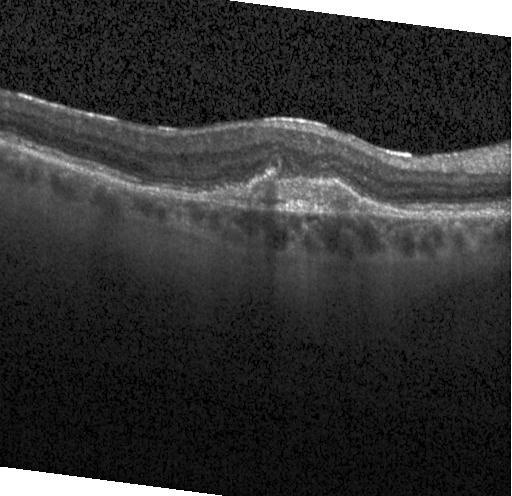
Spectral-domain optical coherence tomography, Heidelberg Spectralis, retinal OCT B-scan — Finding: a choroidal neovascular membrane.